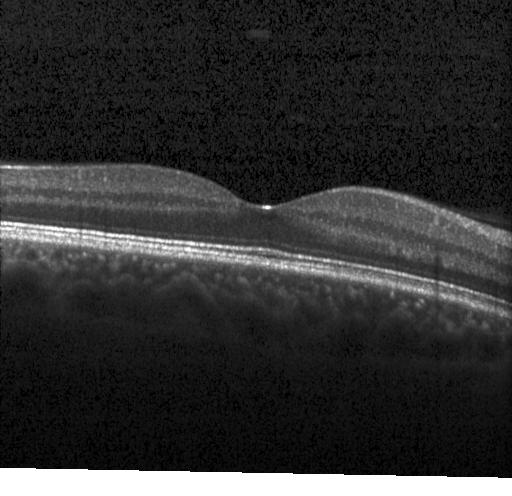 Finding: no choroidal neovascularization, no diabetic macular edema, and no drusen.